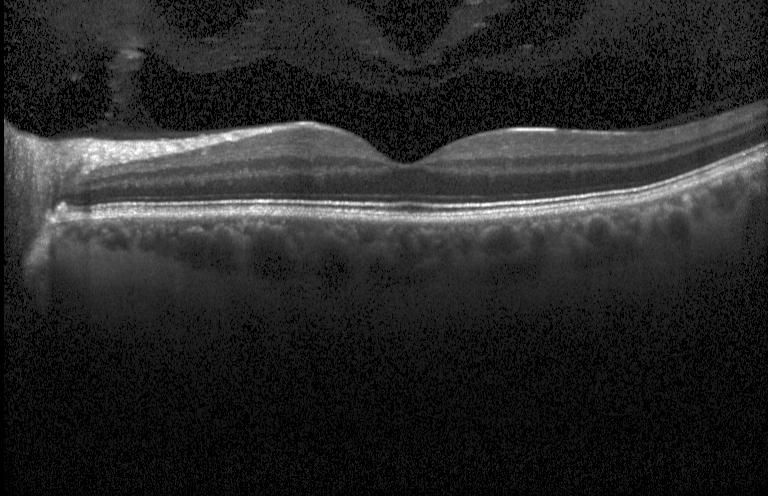 OCT B-scan. Heidelberg Spectralis OCT system
Assessment: no choroidal neovascularization, no diabetic macular edema, and no drusen.